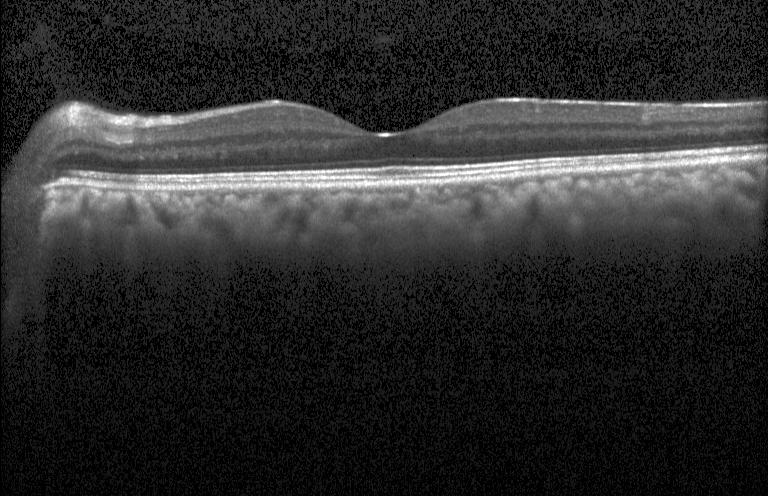
OCT B-scan showing no choroidal neovascularization, diabetic macular edema, or drusen.